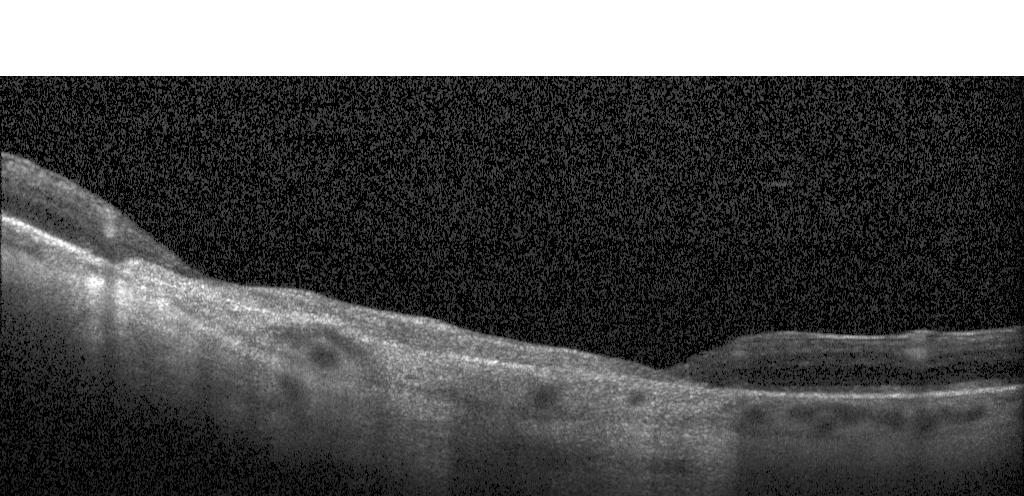

Retinal OCT cross-section. Acquired on a Heidelberg Spectralis
Diagnosis: CNV.